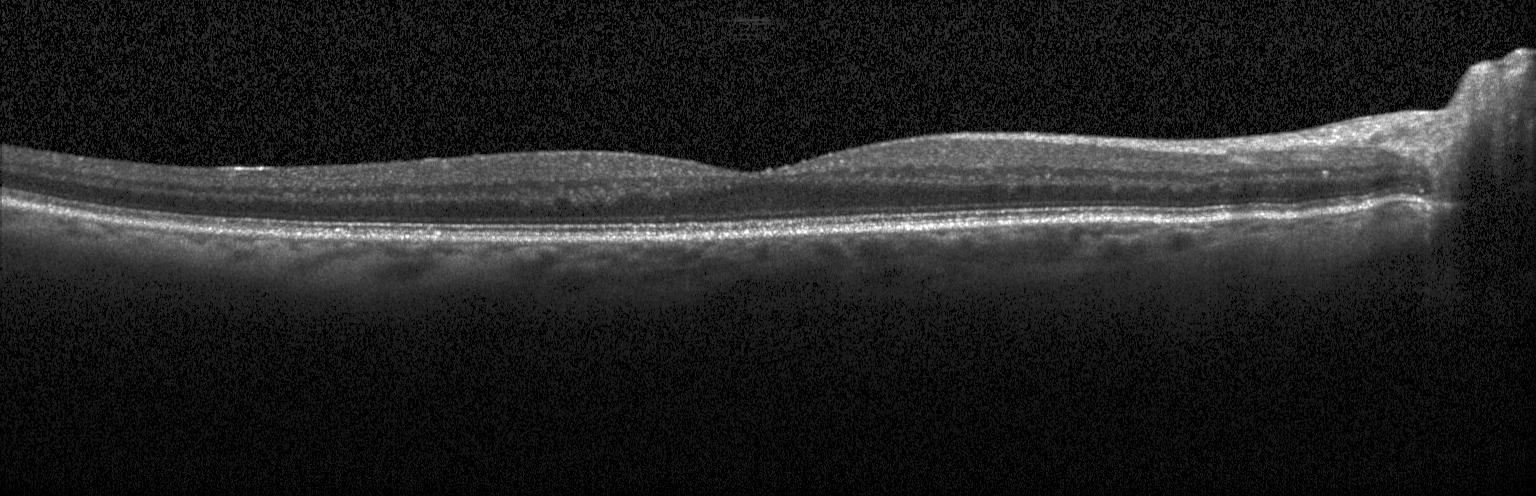

No choroidal neovascularization, diabetic macular edema, or drusen.